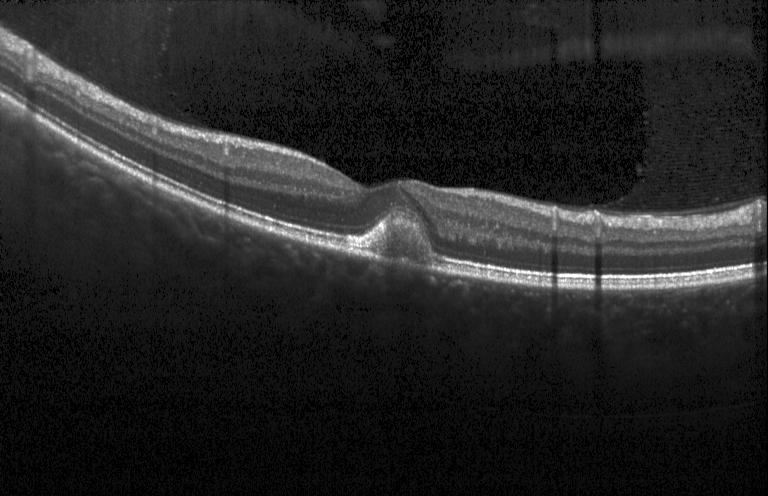 OCT line scan. Diagnosis: sub-RPE drusenoid deposits.